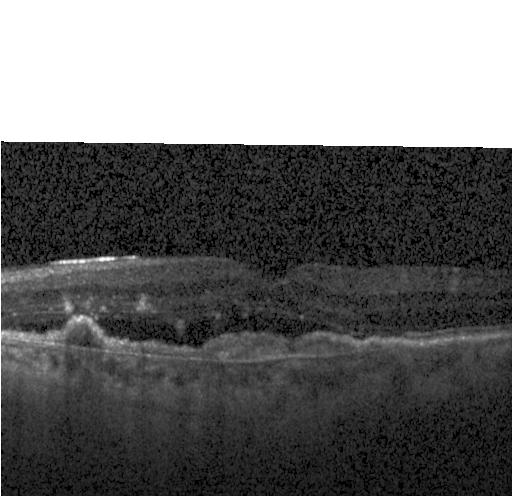

OCT B-scan showing a choroidal neovascular membrane.